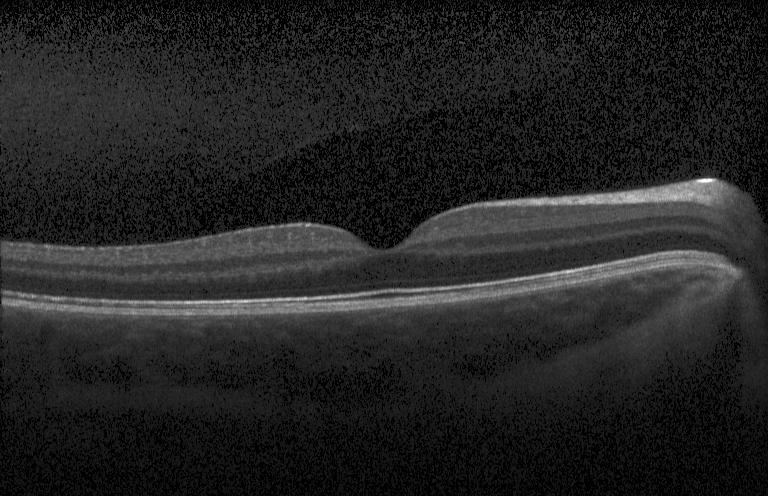
Heidelberg Spectralis OCT system. SD-OCT. OCT line scan. Through the macula.
Dx: neither CNV, DME, nor drusen.